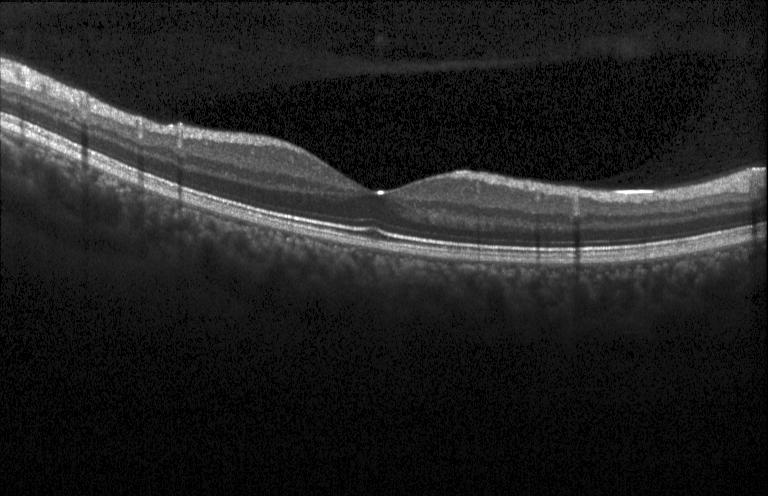 Acquired on a Heidelberg Spectralis. OCT line scan. Assessment: no choroidal neovascularization, no diabetic macular edema, and no drusen.